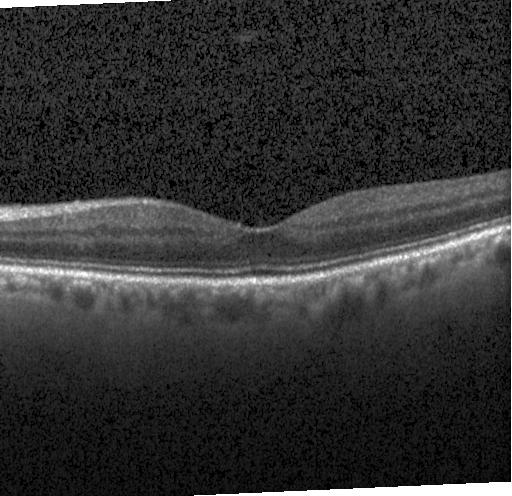 OCT line scan — Finding: no CNV, no DME, and no drusen.